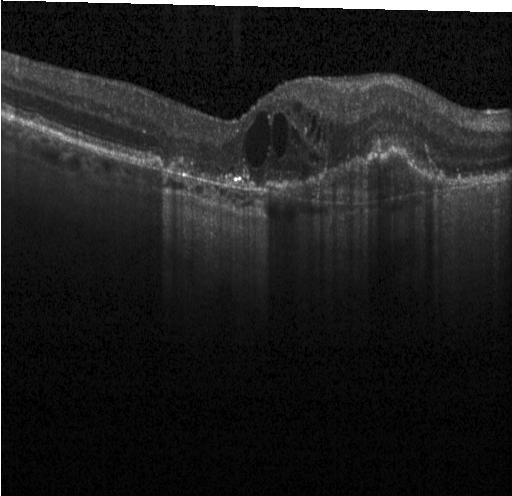 Spectral-domain OCT B-scan: choroidal neovascularization.